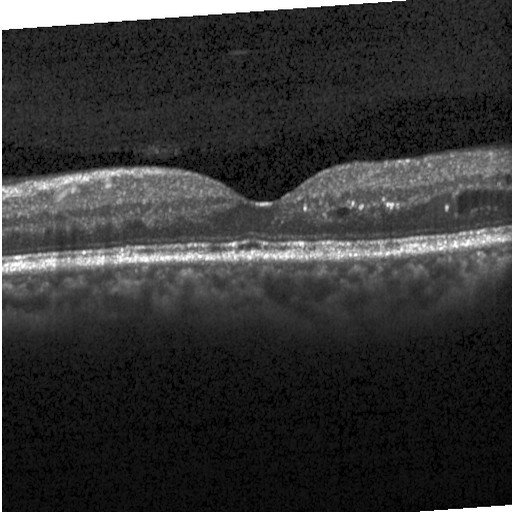 Optical coherence tomography scan · spectral-domain optical coherence tomography. Diagnosis: diabetic macular edema.